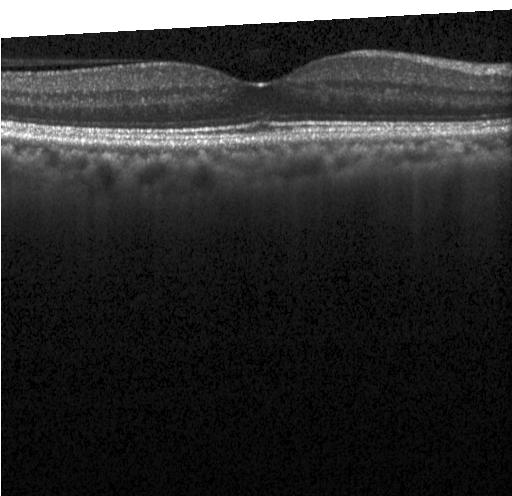

OCT scan showing no choroidal neovascularization, diabetic macular edema, or drusen.